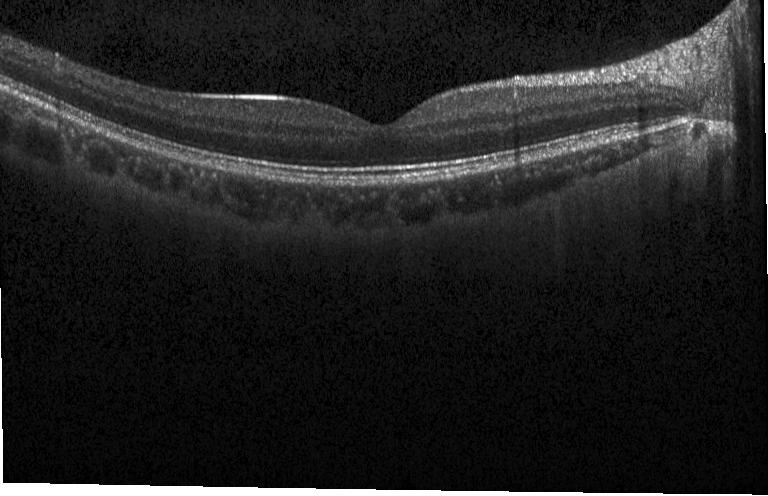

Spectral-domain OCT, optical coherence tomography scan.
Dx: no choroidal neovascularization, diabetic macular edema, or drusen.